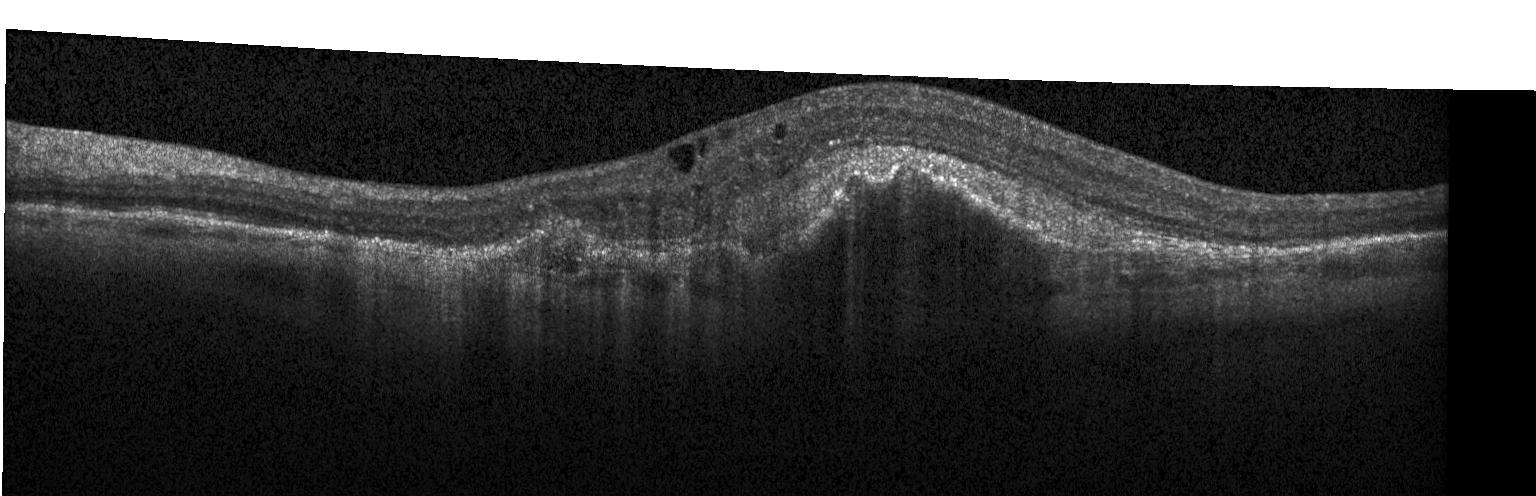
Heidelberg Spectralis. SD-OCT. Horizontal scan through the fovea. Retinal OCT cross-section
This B-scan demonstrates a choroidal neovascular membrane.